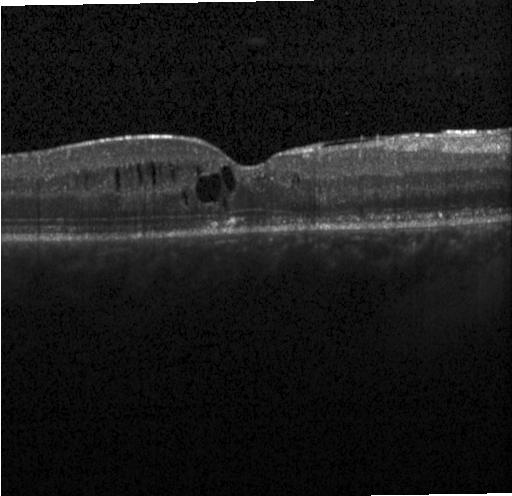 Optical coherence tomography B-scan — Dx: DME.